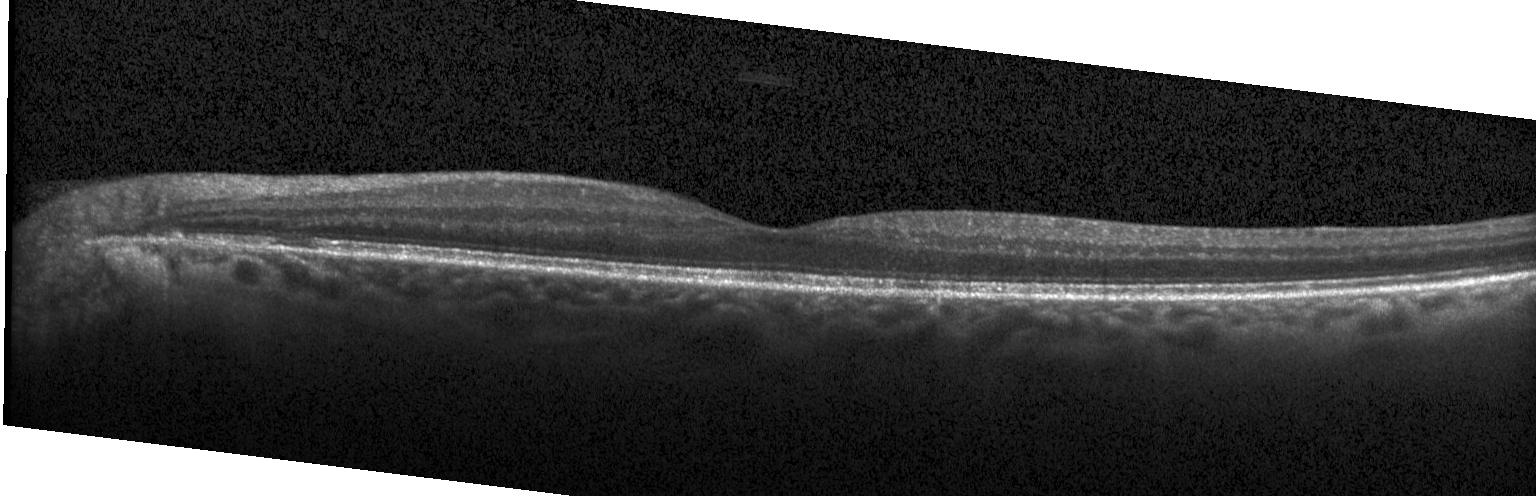
Instrument: Heidelberg Spectralis, SD-OCT, retinal OCT cross-section — Impression: no CNV, DME, or drusen.